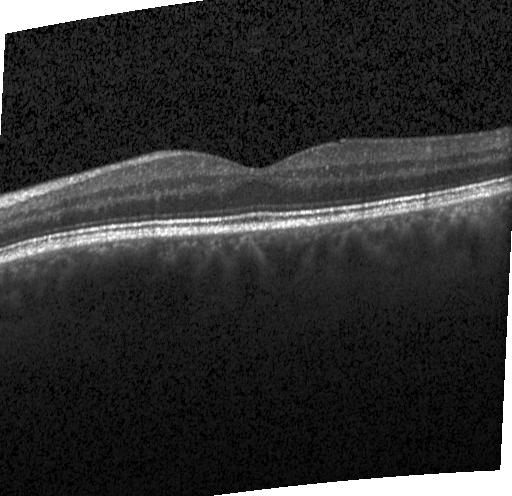 Horizontal scan through the fovea. Spectral-domain optical coherence tomography. Retinal OCT cross-section.
Finding: neither choroidal neovascularization, diabetic macular edema, nor drusen.